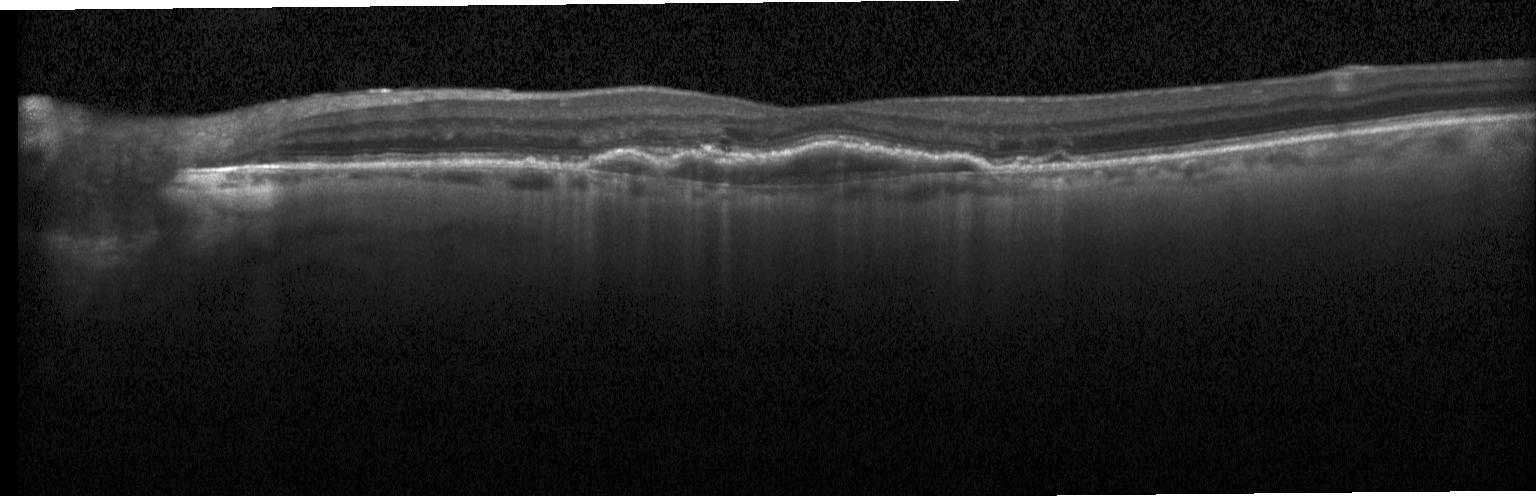

Heidelberg Spectralis · optical coherence tomography scan
Diagnosis: a choroidal neovascular membrane.